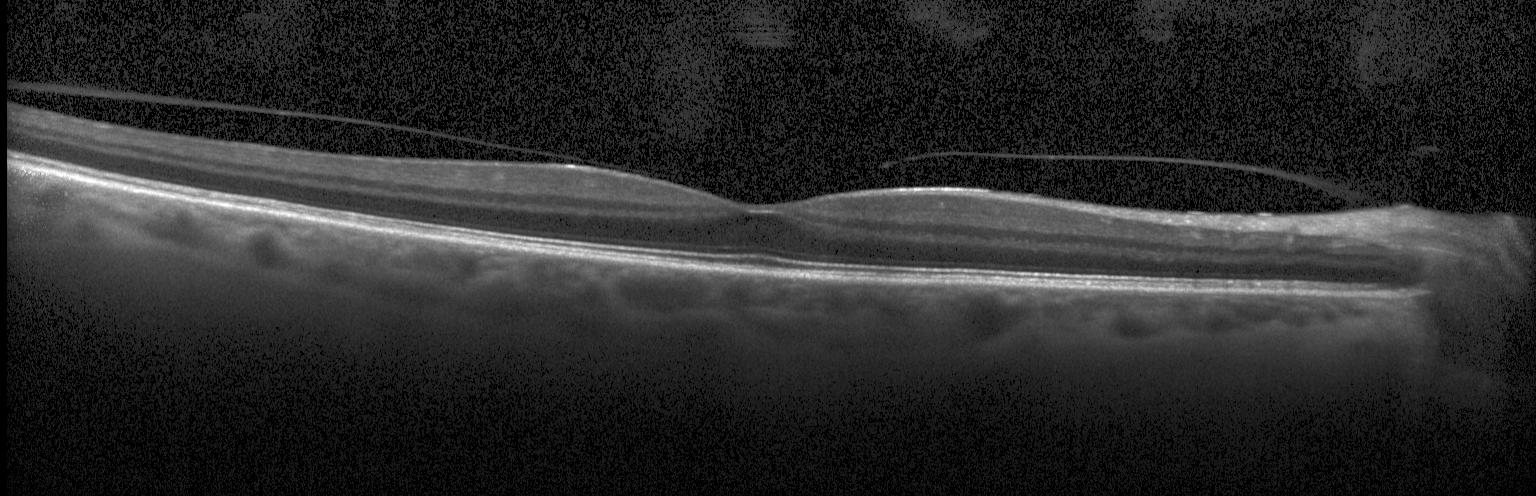

Optical coherence tomography B-scan; spectral-domain optical coherence tomography; Heidelberg Spectralis — Assessment: no choroidal neovascularization, diabetic macular edema, or drusen.